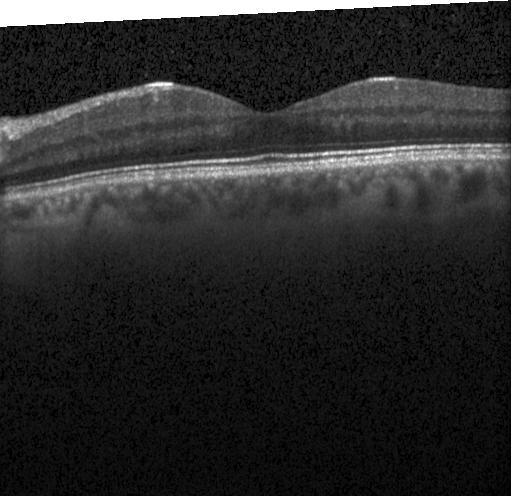

Retinal OCT cross-section showing no choroidal neovascularization, no diabetic macular edema, and no drusen.